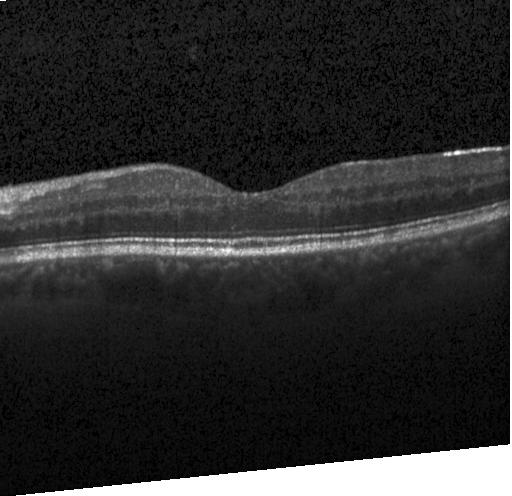

Macular scan; retinal OCT B-scan. Assessment: no choroidal neovascularization, diabetic macular edema, or drusen.